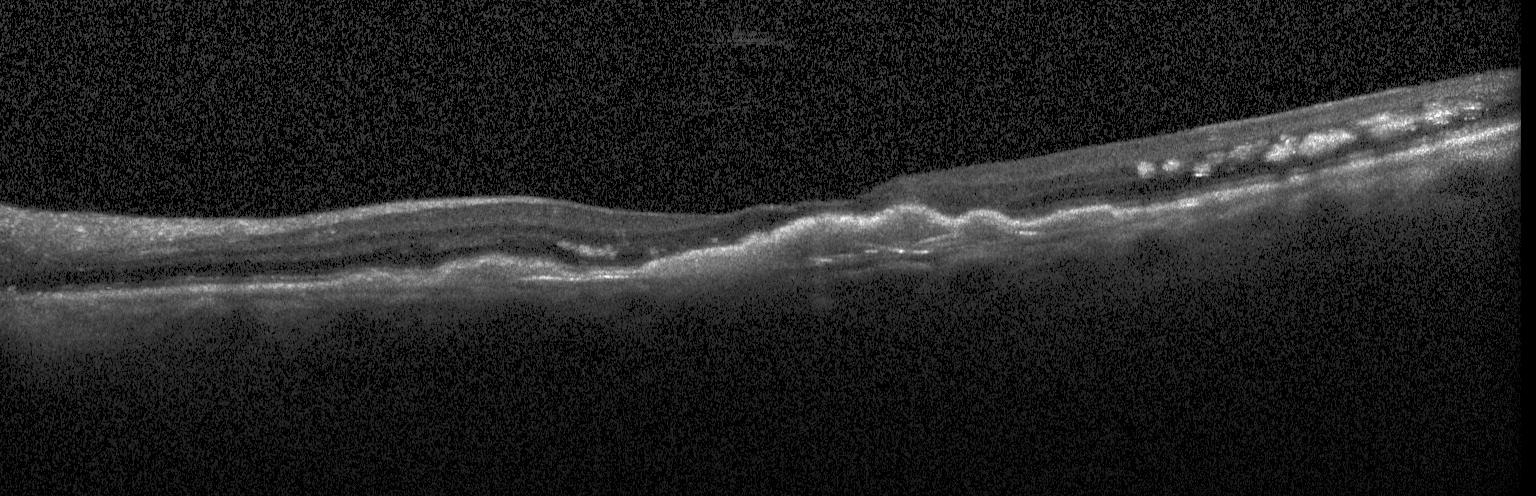

Diagnosis: a choroidal neovascular membrane.